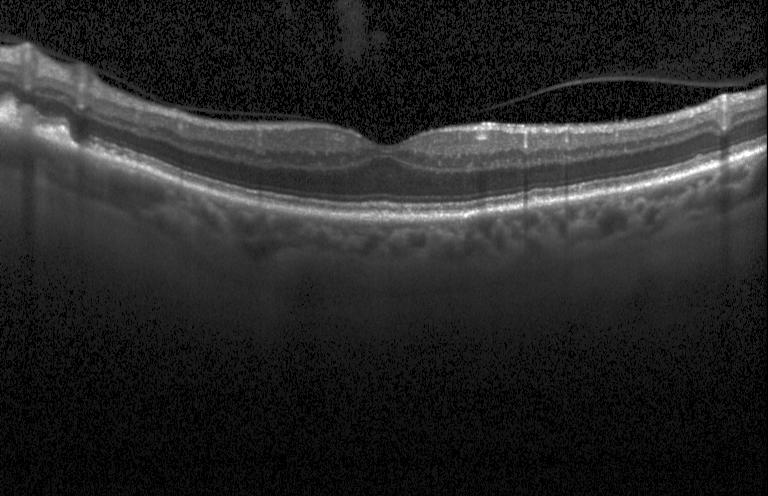
Finding: no evidence of CNV, DME, or drusen.